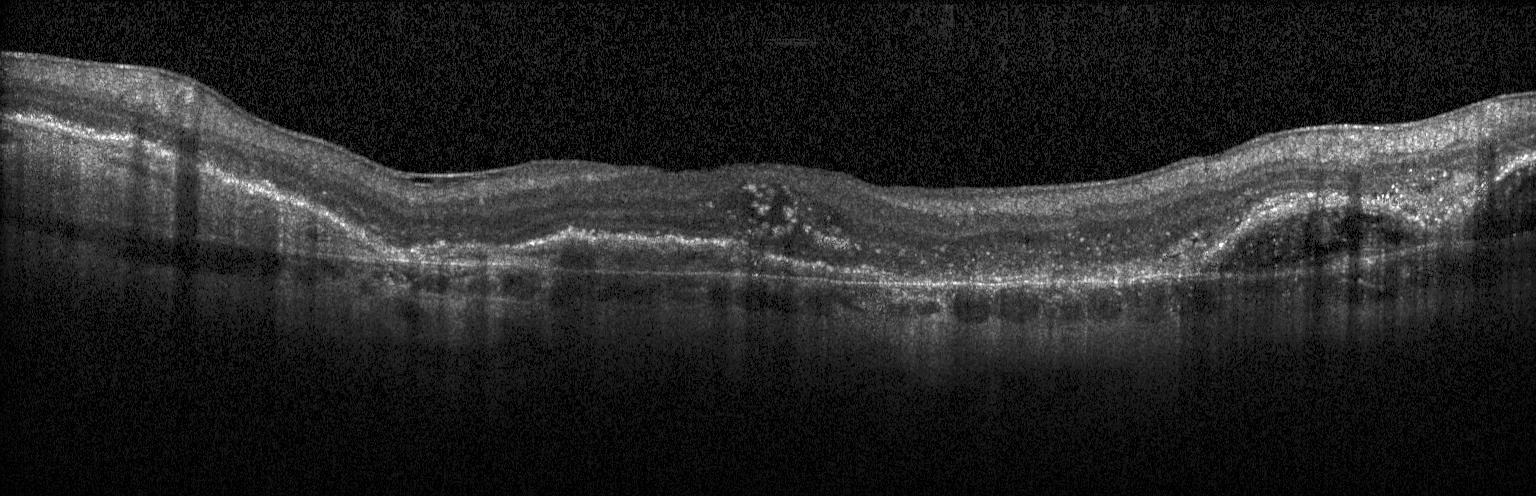 SD-OCT; centered on the fovea; Heidelberg Spectralis OCT system; retinal OCT B-scan — Impression: a choroidal neovascular membrane.